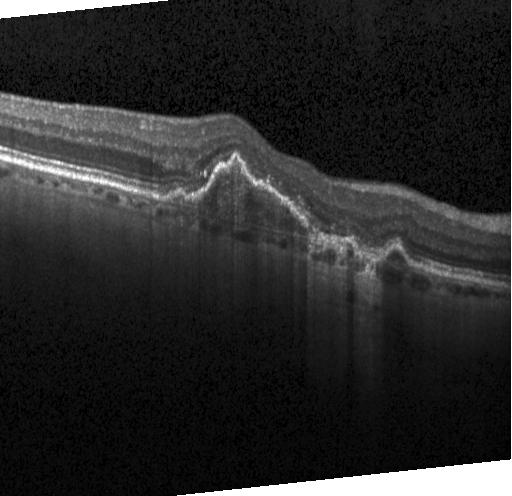 Spectral-domain OCT; centered on the fovea; acquired on a Heidelberg Spectralis; retinal OCT B-scan. Diagnosis: a choroidal neovascular membrane.